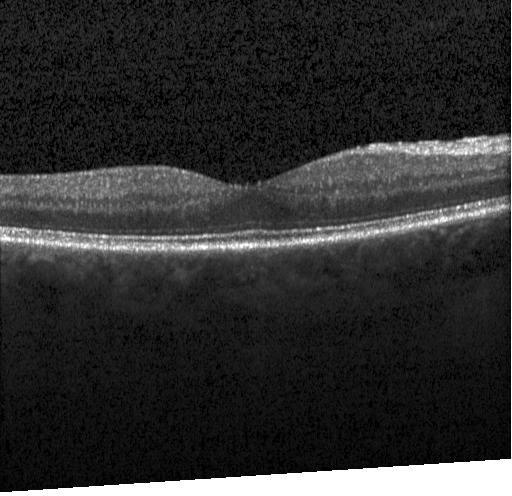 Centered on the fovea. Retinal OCT cross-section. Finding: neither choroidal neovascularization, diabetic macular edema, nor drusen.